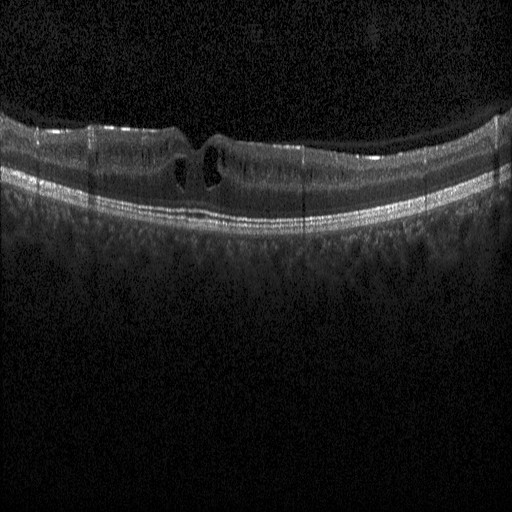 Spectral-domain OCT; optical coherence tomography scan. Impression: diabetic macular edema (DME).